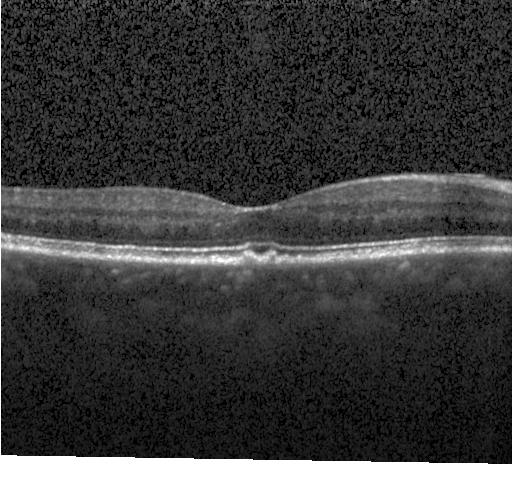

Spectral-domain optical coherence tomography · OCT line scan · Heidelberg Spectralis · horizontal scan through the fovea. Finding: sub-RPE drusenoid deposits.